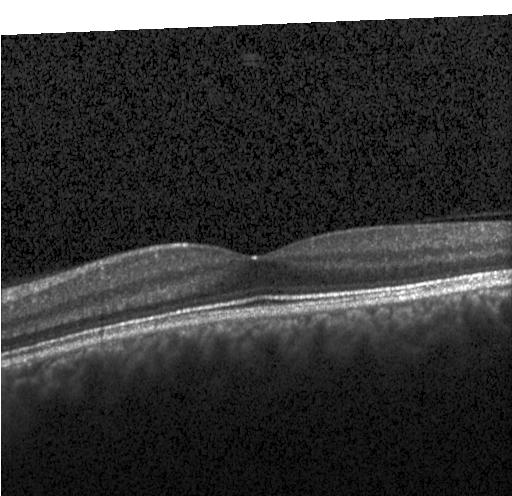
Finding: neither choroidal neovascularization, diabetic macular edema, nor drusen.